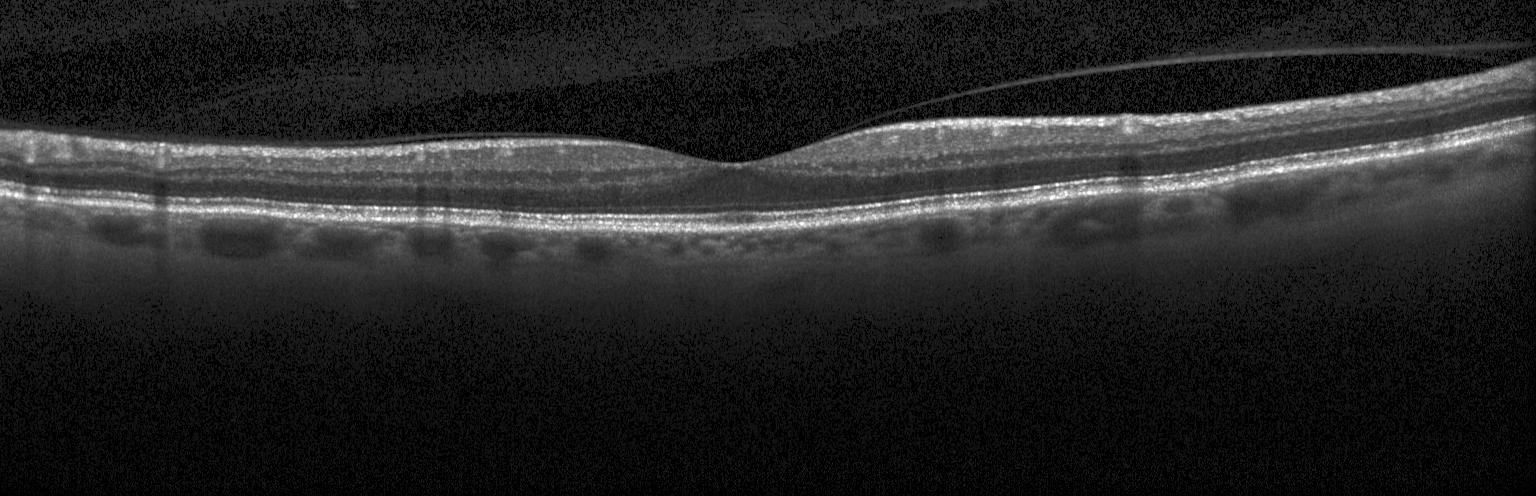 OCT B-scan showing no CNV, DME, or drusen.